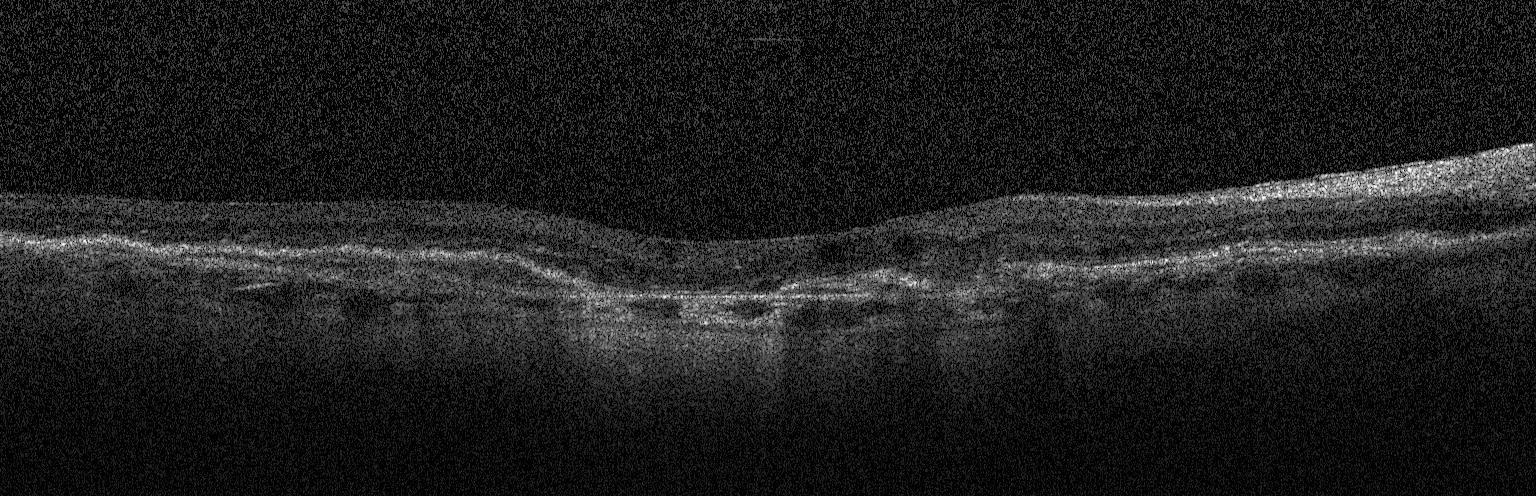 OCT B-scan showing a choroidal neovascular membrane.